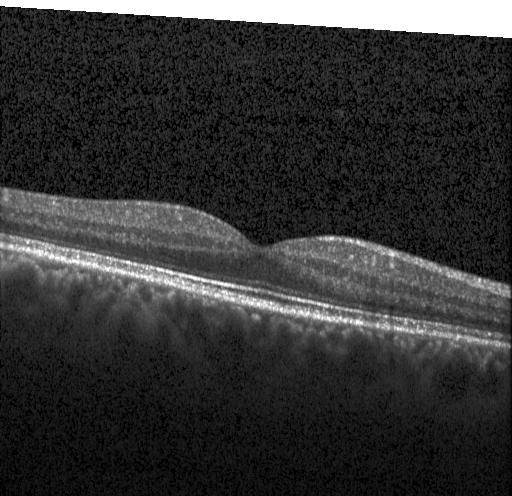
OCT line scan.
Macular OCT: no choroidal neovascularization, diabetic macular edema, or drusen.